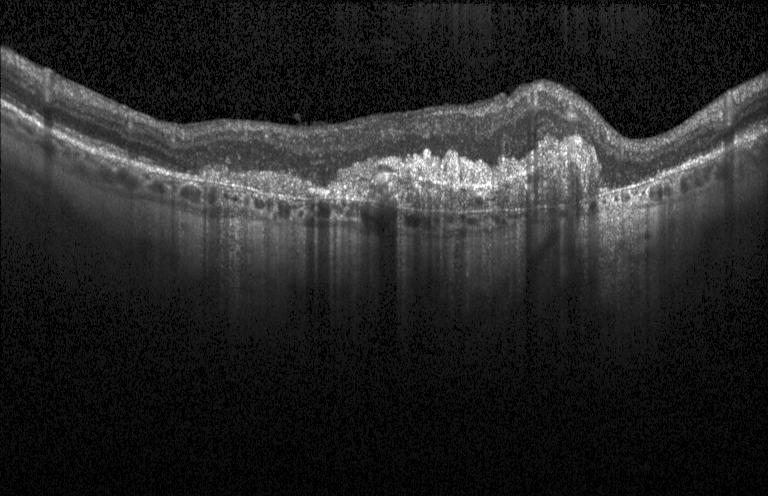

OCT scan showing CNV.